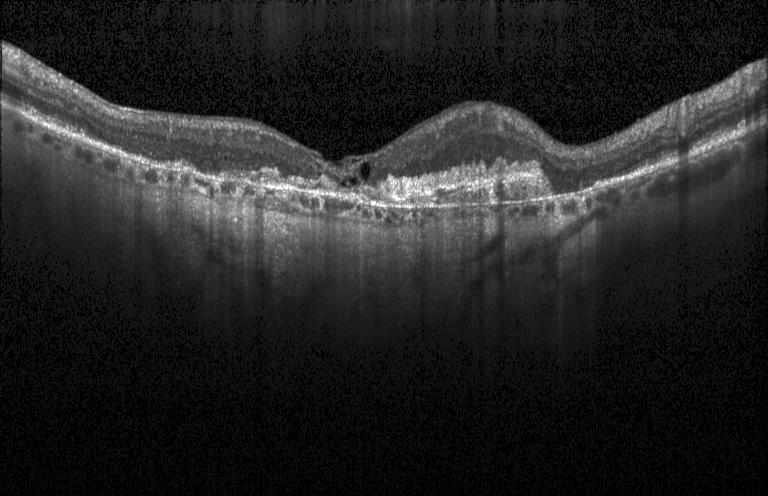

Diagnosis: a choroidal neovascular membrane.